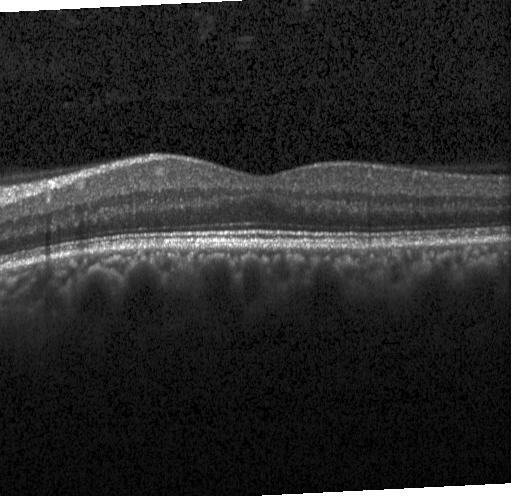 Impression: neither choroidal neovascularization, diabetic macular edema, nor drusen.